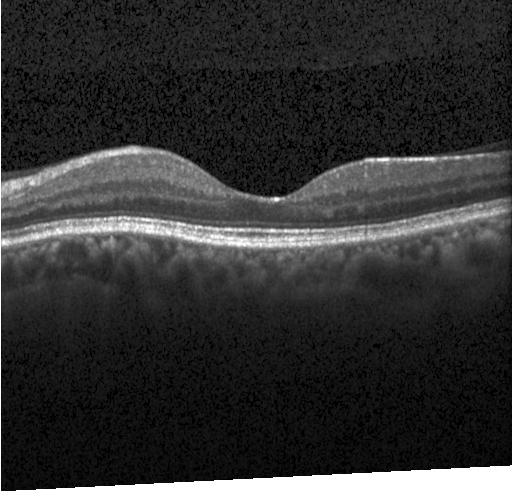

Optical coherence tomography B-scan, SD-OCT, horizontal scan through the fovea, Heidelberg Spectralis OCT system — Diagnosis: no choroidal neovascularization, diabetic macular edema, or drusen.